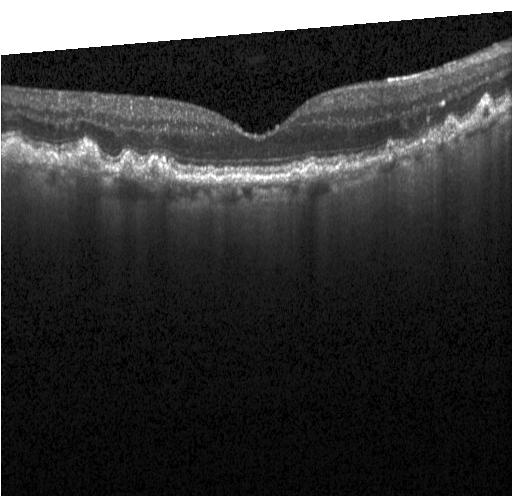
Diagnosis: multiple drusen.